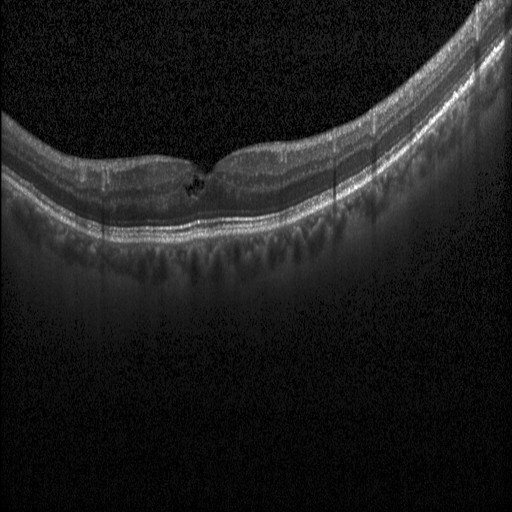 Heidelberg Spectralis OCT system, OCT B-scan.
Assessment: diabetic macular edema (DME).